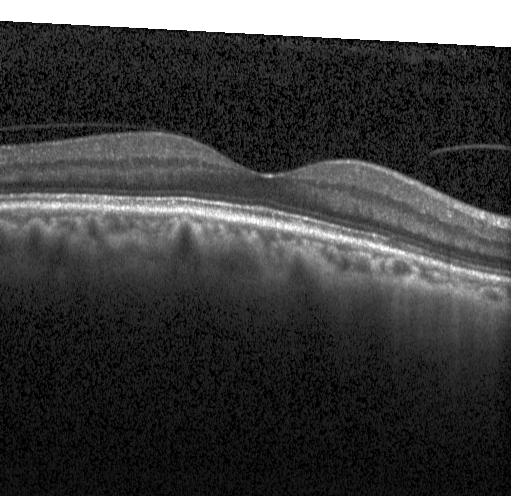
Optical coherence tomography scan.
OCT finding: neither choroidal neovascularization, diabetic macular edema, nor drusen.